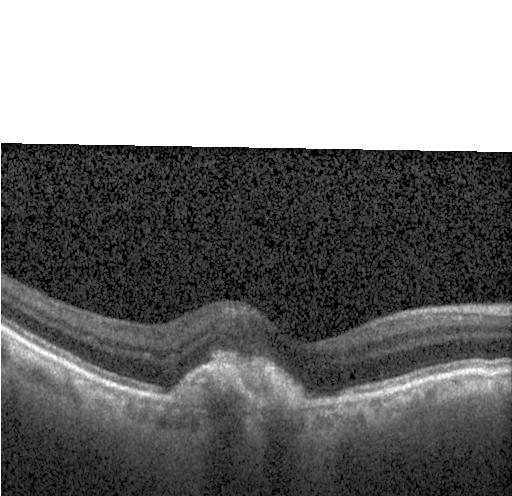

Instrument: Heidelberg Spectralis · SD-OCT · through the macula · retinal OCT B-scan
Macular OCT: a choroidal neovascular membrane.